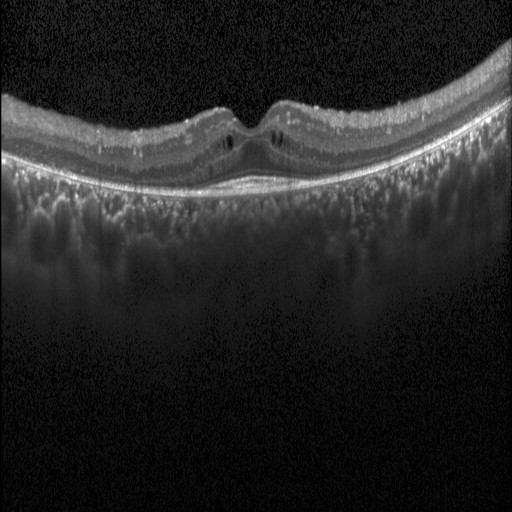 Finding: DME.